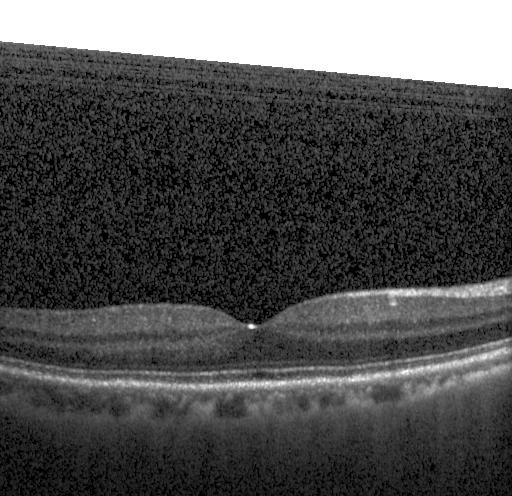
Macular OCT: no evidence of choroidal neovascularization, diabetic macular edema, or drusen.